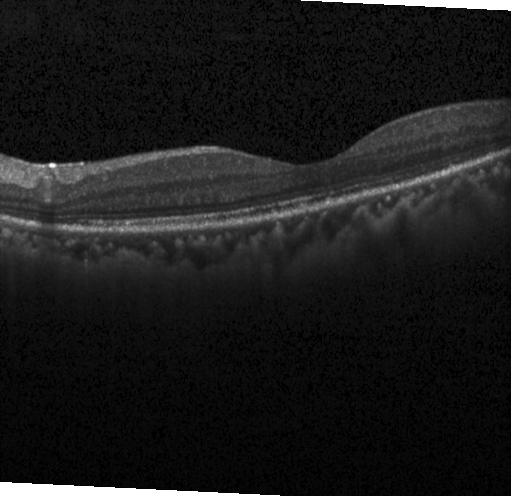
OCT line scan. Spectral-domain OCT. Macular scan — OCT finding: neither choroidal neovascularization, diabetic macular edema, nor drusen.